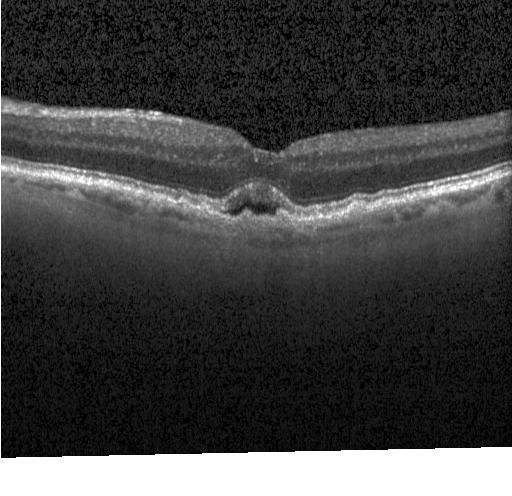

Diagnosis: a choroidal neovascular membrane.